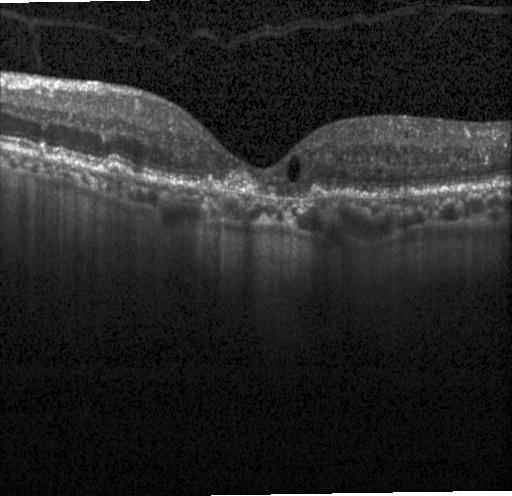 Optical coherence tomography B-scan. Horizontal scan through the fovea — This B-scan demonstrates a choroidal neovascular membrane.